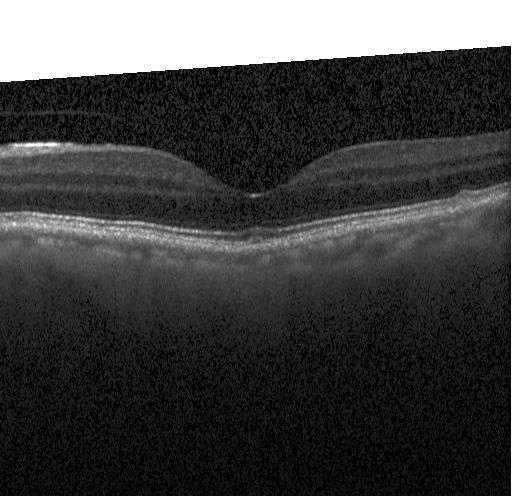 Spectral-domain OCT, Heidelberg Spectralis, optical coherence tomography scan. Impression: neither choroidal neovascularization, diabetic macular edema, nor drusen.